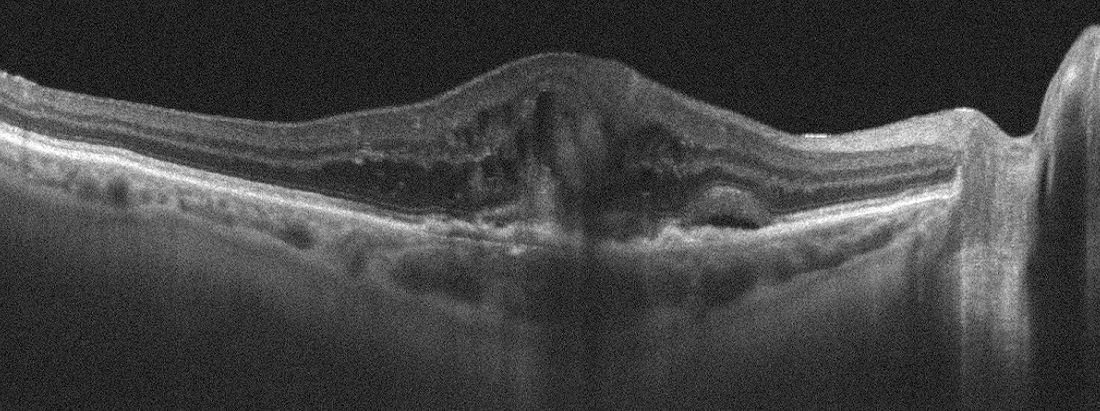

Through the macula · Optovue Avanti RTVue XR · optical coherence tomography scan. Finding: age-related macular degeneration.